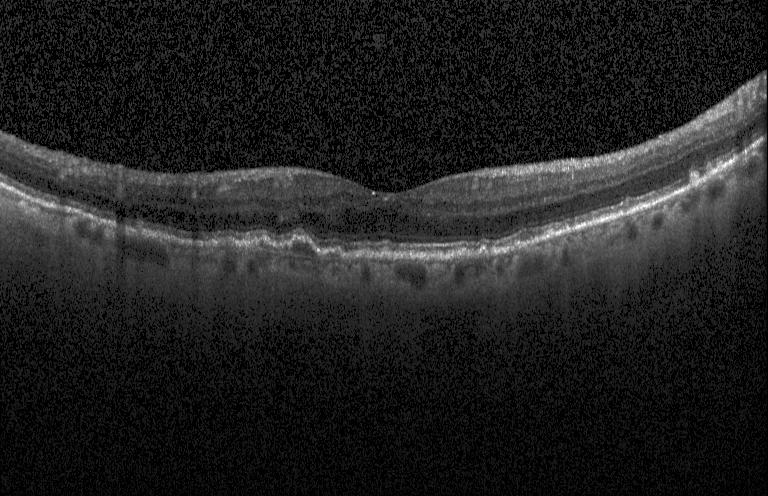 Finding: drusen.